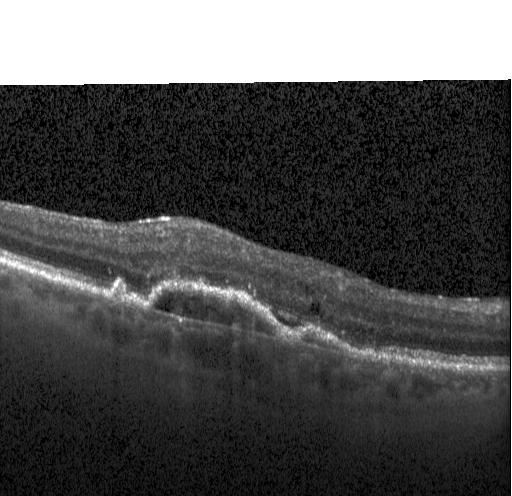

Fovea-centered · acquired on a Heidelberg Spectralis · spectral-domain OCT · retinal OCT cross-section — Assessment: choroidal neovascularization (CNV).